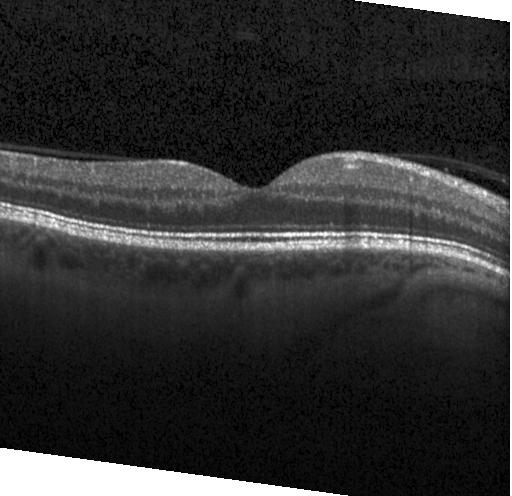 Through the macula; optical coherence tomography B-scan — The scan shows no choroidal neovascularization, no diabetic macular edema, and no drusen.